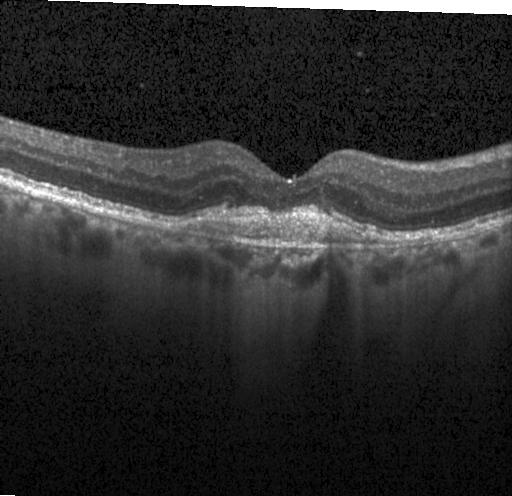

Fovea-centered, retinal OCT B-scan, instrument: Heidelberg Spectralis. This B-scan demonstrates choroidal neovascularization.